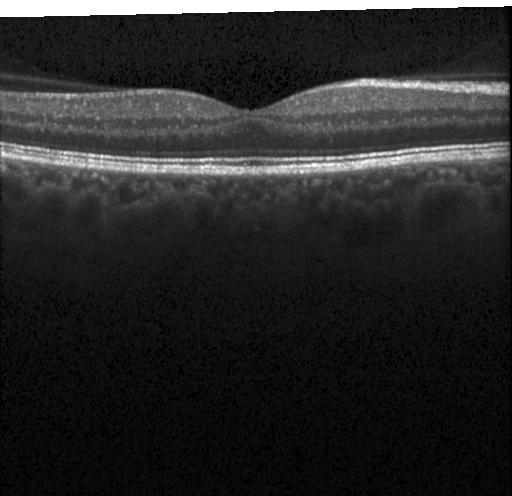
Instrument: Heidelberg Spectralis. SD-OCT. OCT line scan. Macular scan. This B-scan demonstrates no evidence of CNV, DME, or drusen.